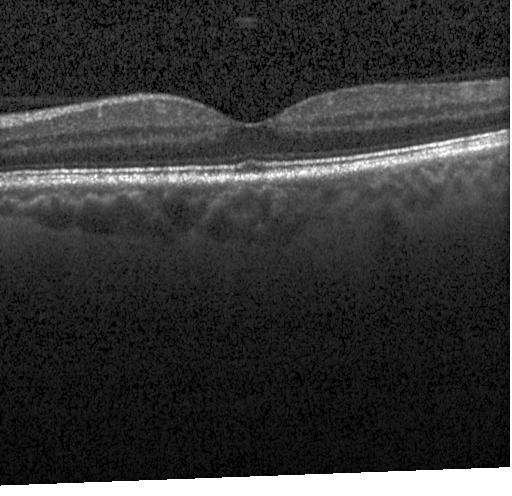
OCT line scan
Finding: no evidence of choroidal neovascularization, diabetic macular edema, or drusen.